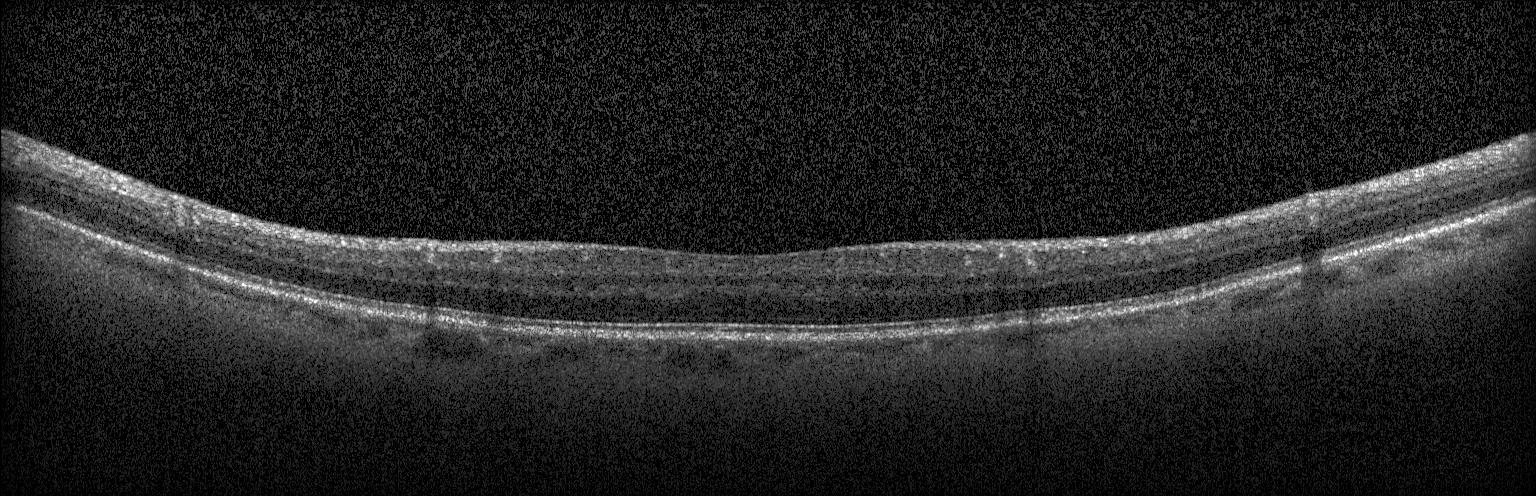
Impression: neither choroidal neovascularization, diabetic macular edema, nor drusen.